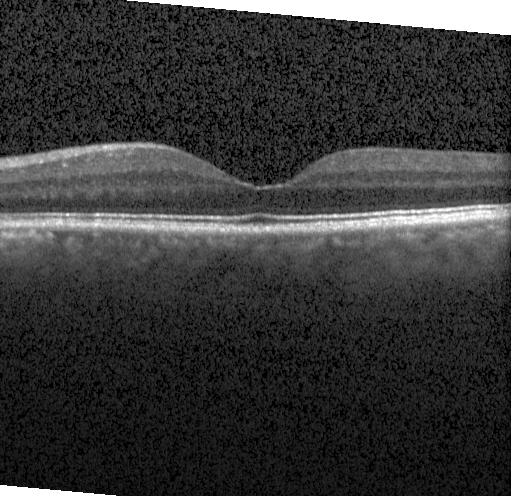

Macular scan, OCT B-scan. This B-scan demonstrates no choroidal neovascularization, diabetic macular edema, or drusen.